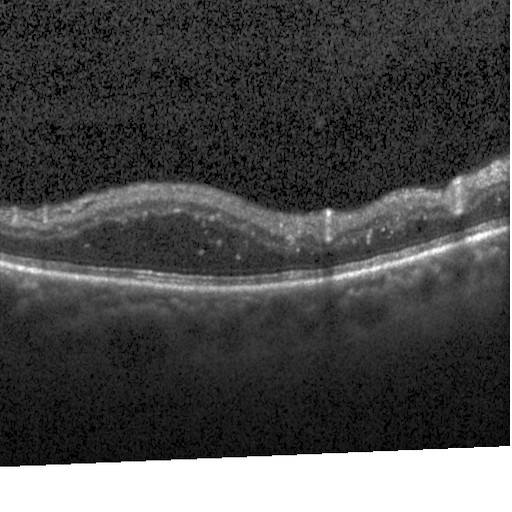

Fovea-centered · retinal OCT cross-section — Finding: diabetic macular edema (DME).